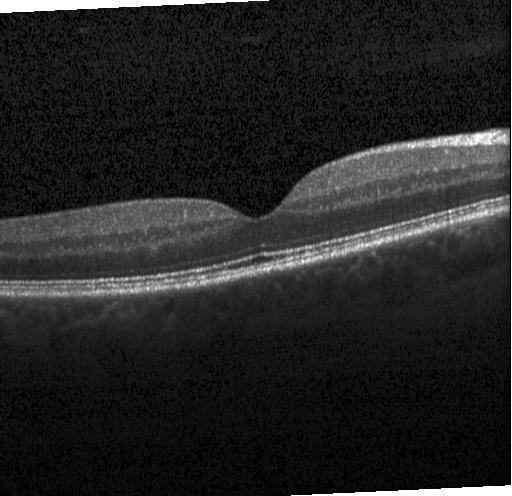
Instrument: Heidelberg Spectralis, optical coherence tomography B-scan, spectral-domain OCT — Assessment: no choroidal neovascularization, diabetic macular edema, or drusen.